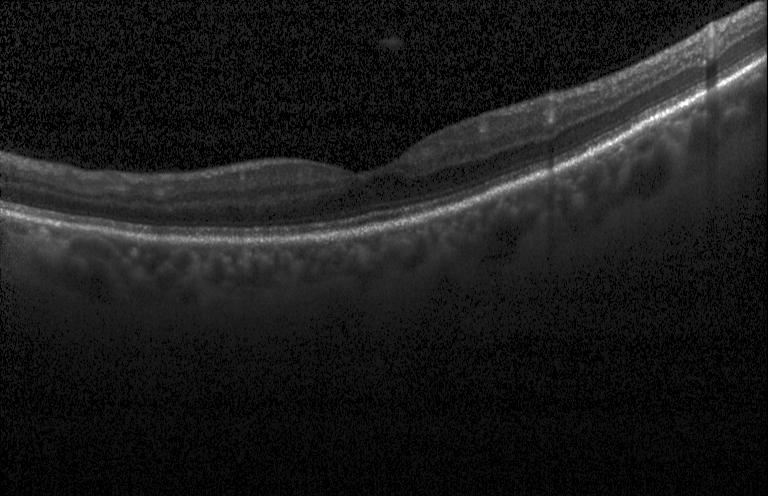 This B-scan demonstrates no CNV, DME, or drusen.